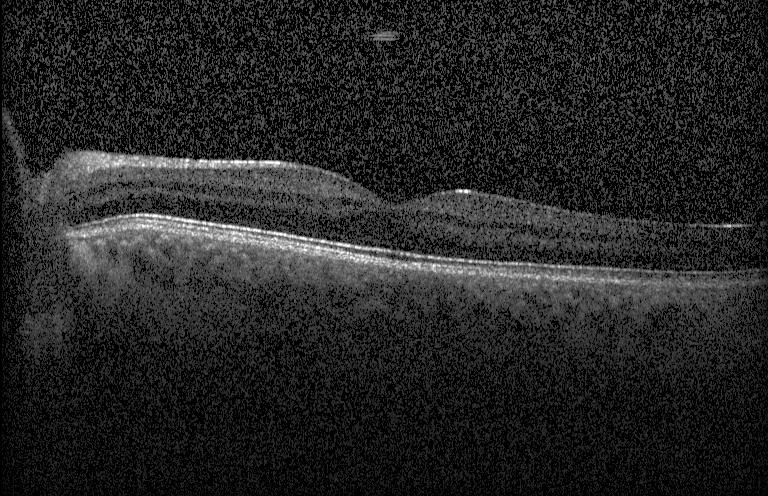 Heidelberg Spectralis; through the macula; retinal OCT cross-section; SD-OCT — This B-scan demonstrates neither CNV, DME, nor drusen.